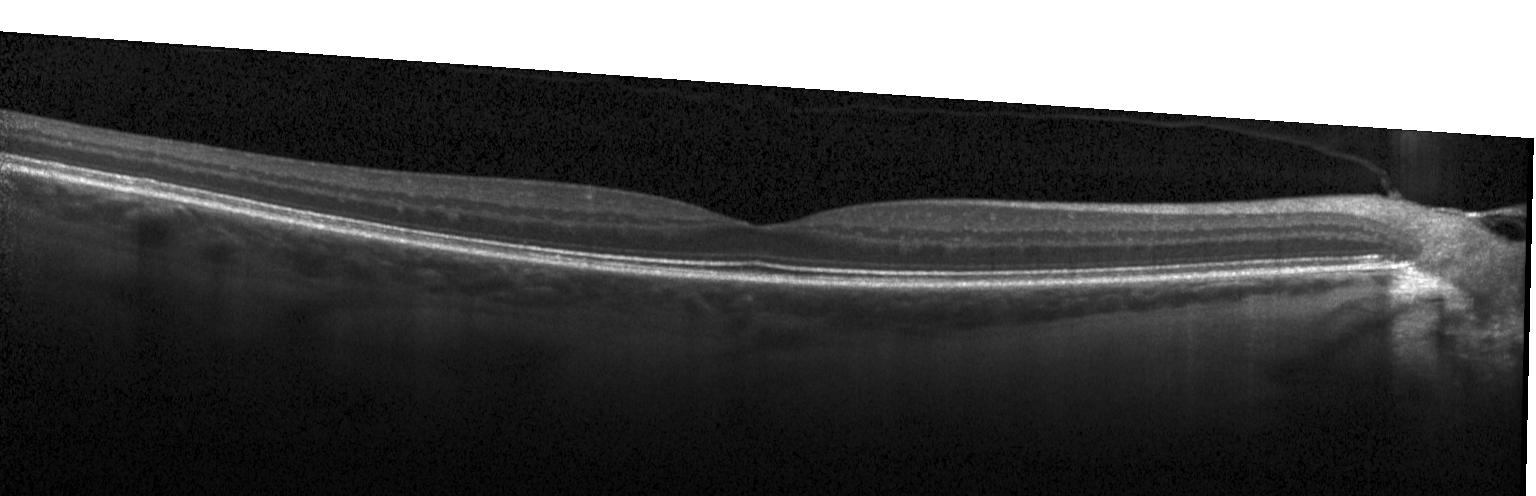 OCT finding: neither choroidal neovascularization, diabetic macular edema, nor drusen.